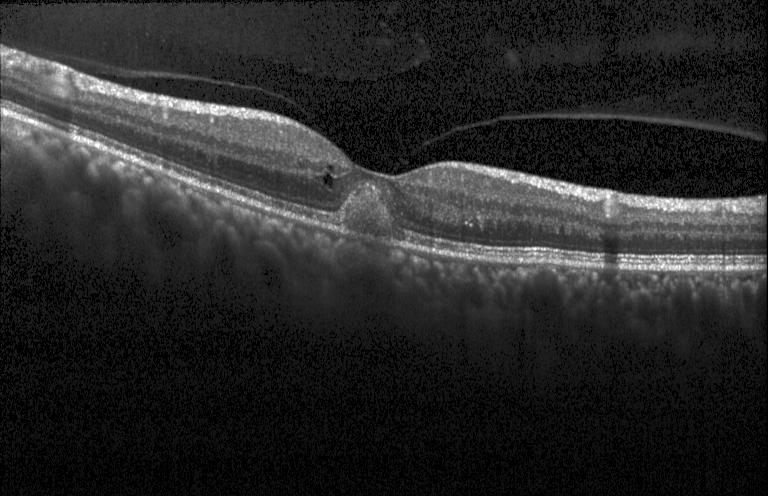
OCT B-scan; acquired on a Heidelberg Spectralis; SD-OCT; through the macula
Impression: choroidal neovascularization.